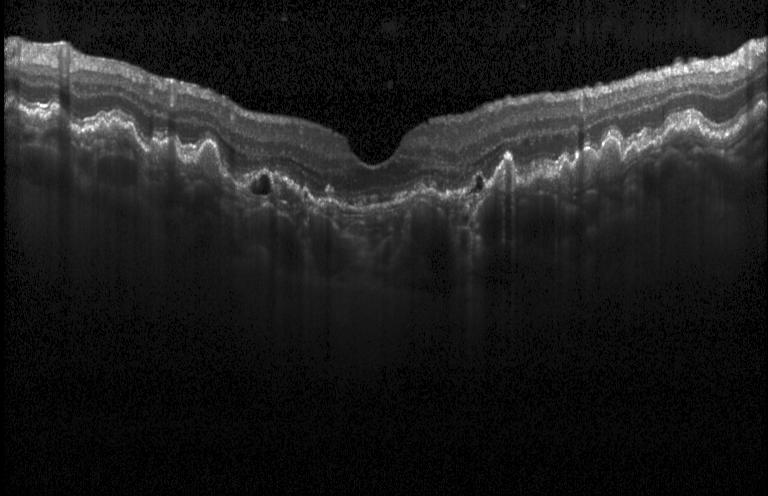
Instrument: Heidelberg Spectralis; OCT line scan; SD-OCT; centered on the fovea.
Finding: a choroidal neovascular membrane.